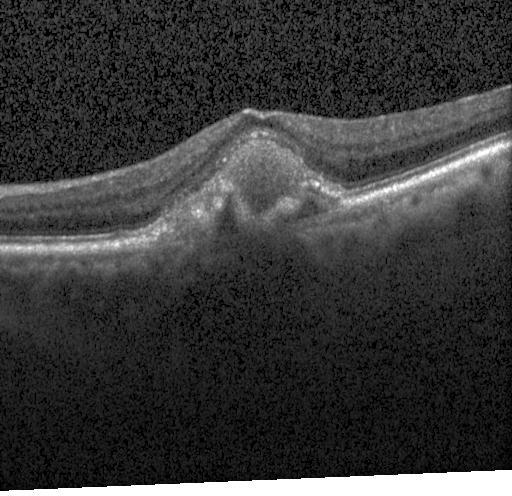 Assessment: a choroidal neovascular membrane.